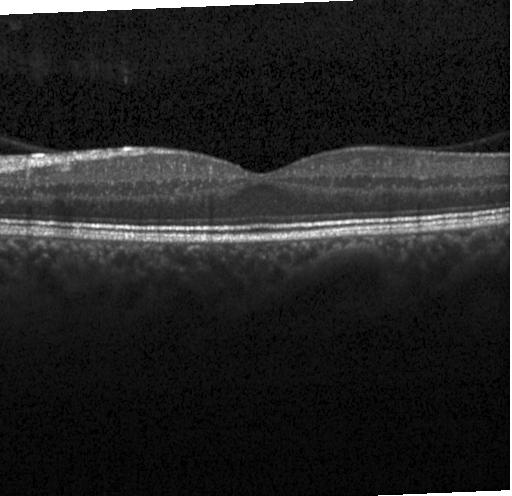
OCT finding: neither choroidal neovascularization, diabetic macular edema, nor drusen.